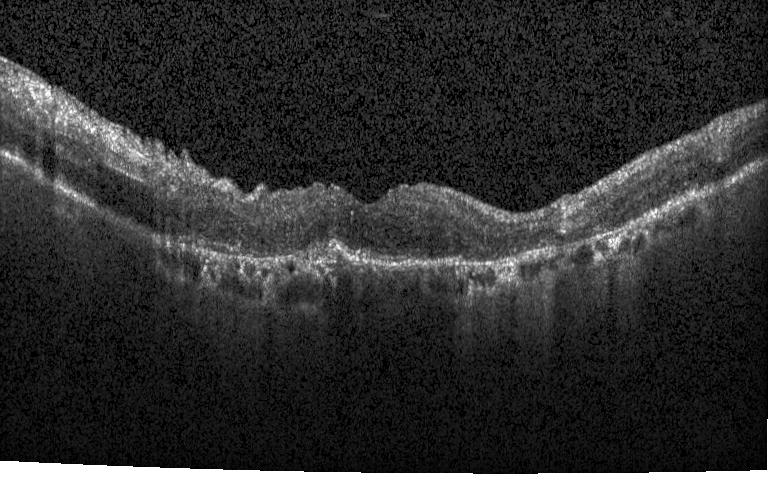 Through the macula; OCT line scan. Impression: CNV.